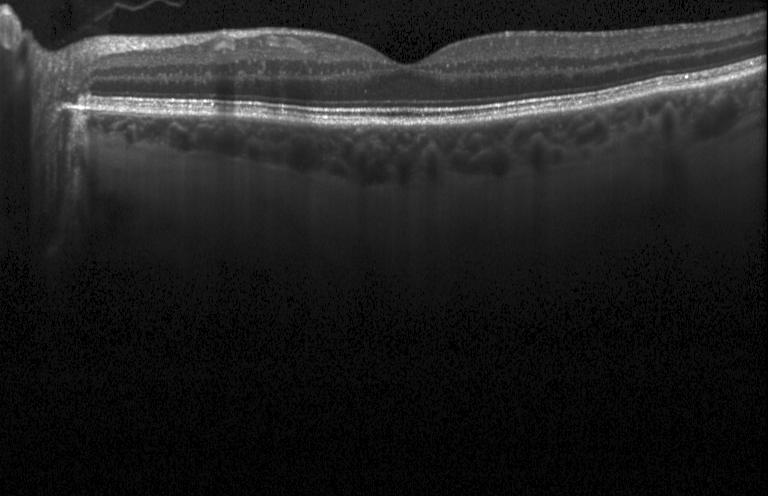

Optical coherence tomography scan. Spectral-domain OCT. Instrument: Heidelberg Spectralis. Fovea-centered.
OCT finding: no choroidal neovascularization, diabetic macular edema, or drusen.